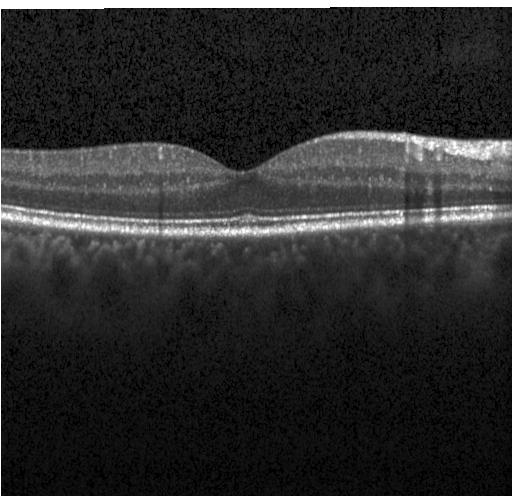 Retinal OCT B-scan
Diagnosis: no evidence of choroidal neovascularization, diabetic macular edema, or drusen.